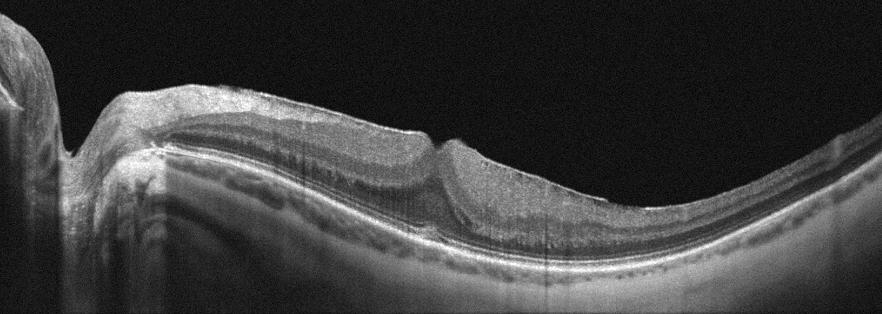
OS; retinal OCT cross-section
Assessment: epiretinal membrane (ERM).